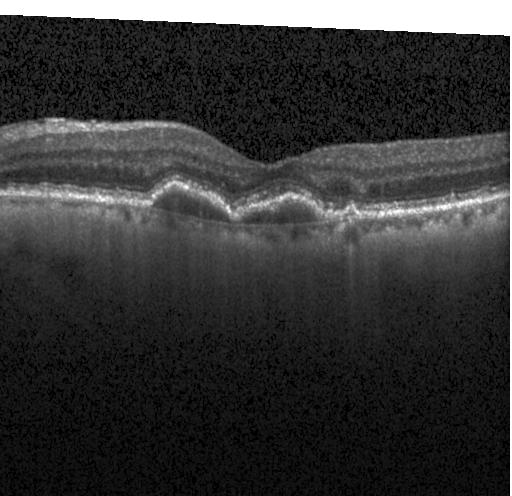
Retinal OCT B-scan · spectral-domain OCT
This B-scan demonstrates choroidal neovascularization.